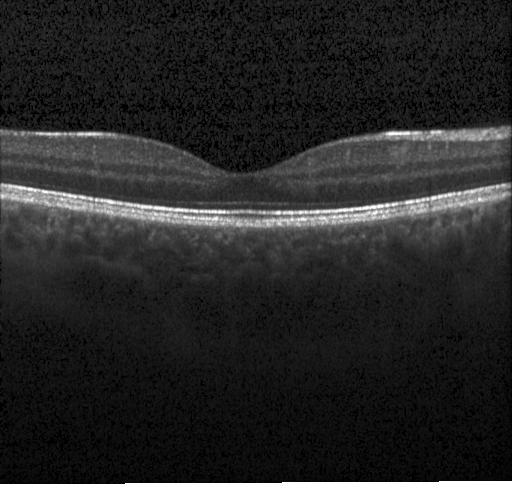 Spectral-domain OCT; optical coherence tomography B-scan; Heidelberg Spectralis; through the macula. Diagnosis: no CNV, DME, or drusen.